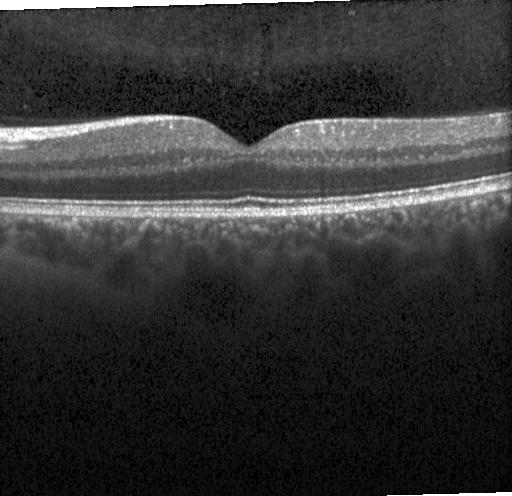
Impression: no choroidal neovascularization, diabetic macular edema, or drusen.